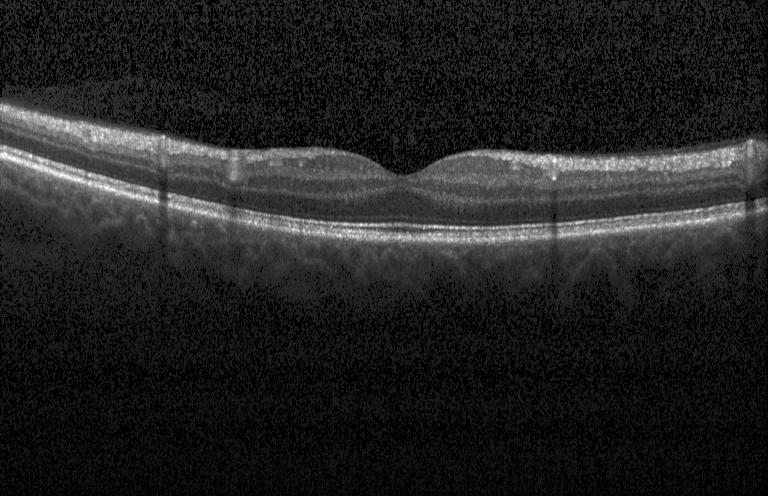
Retinal OCT cross-section; Heidelberg Spectralis OCT system; spectral-domain OCT — No CNV, DME, or drusen.